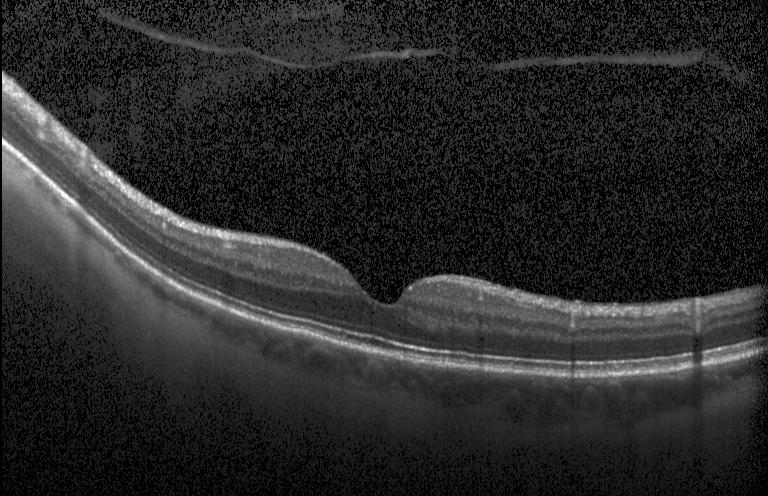
OCT B-scan
Finding: no evidence of choroidal neovascularization, diabetic macular edema, or drusen.